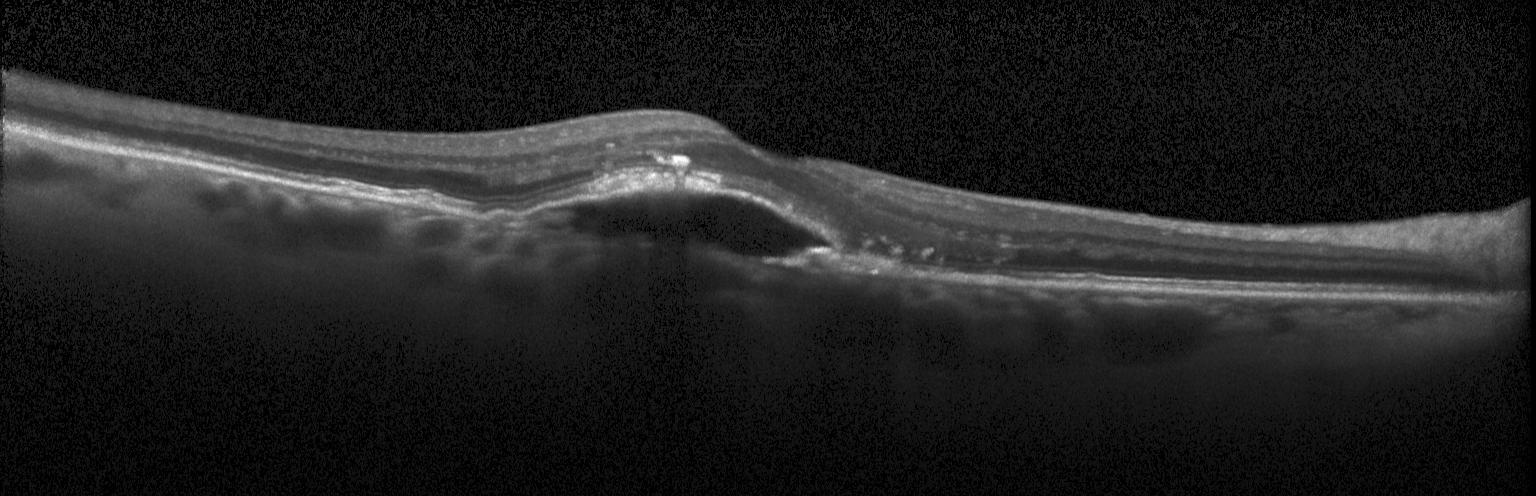

Diagnosis: a choroidal neovascular membrane.